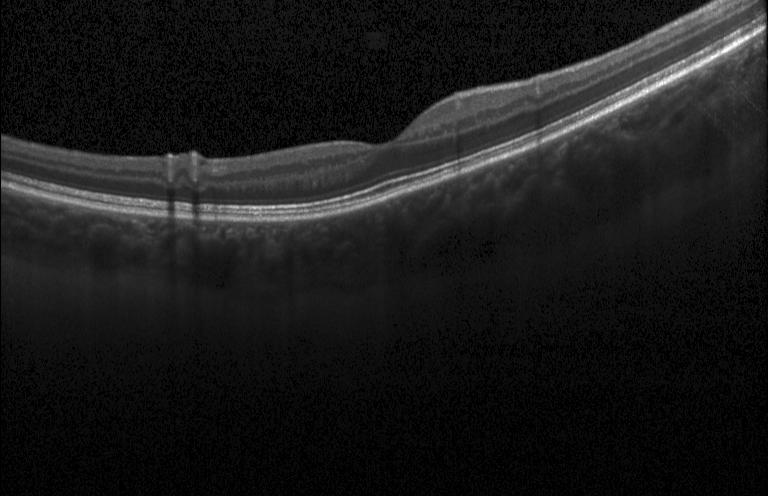 OCT line scan; centered on the fovea; Heidelberg Spectralis OCT system; spectral-domain OCT.
Dx: no evidence of CNV, DME, or drusen.